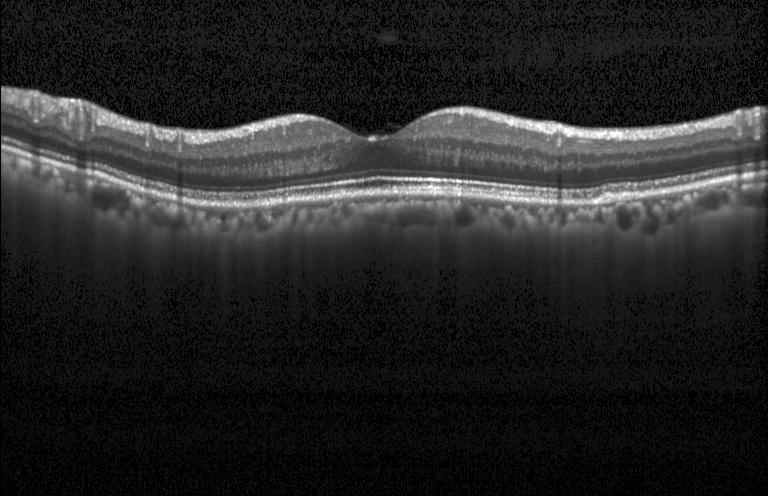 OCT B-scan showing no choroidal neovascularization, no diabetic macular edema, and no drusen.